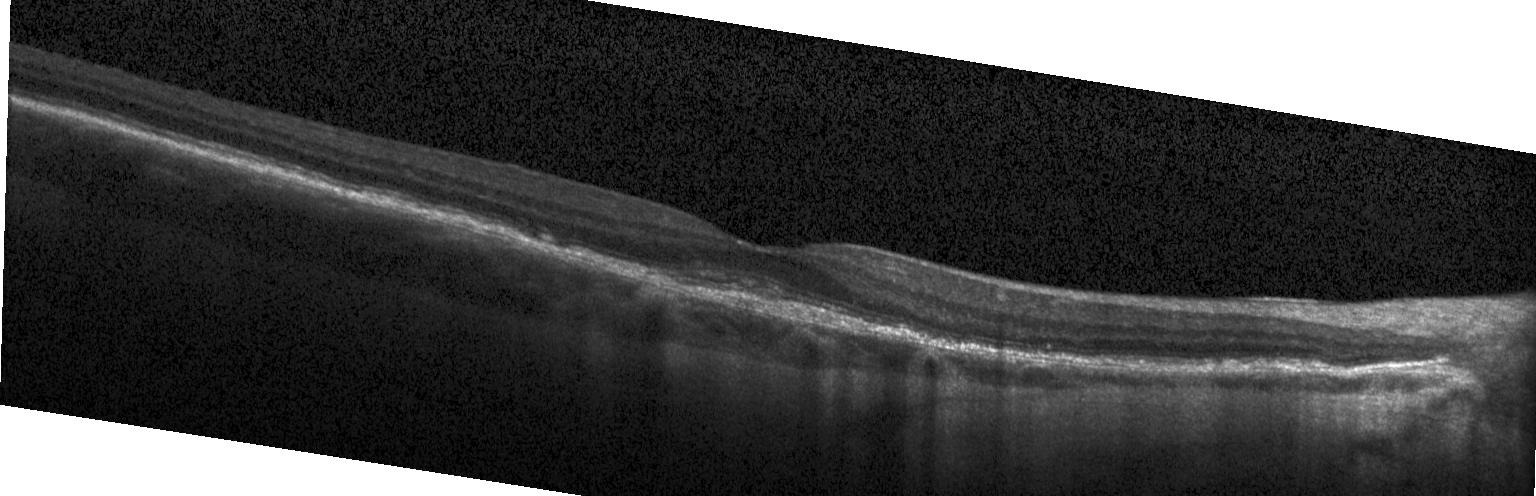

Impression: a choroidal neovascular membrane.